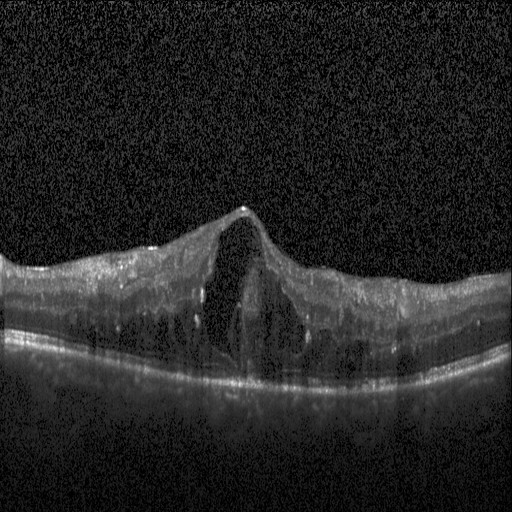

This B-scan demonstrates diabetic macular edema.